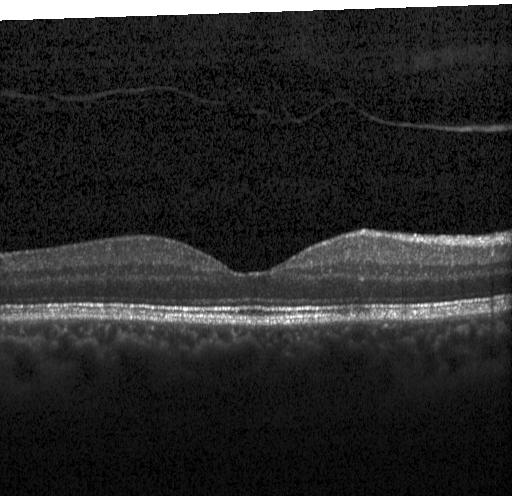

The scan shows no evidence of CNV, DME, or drusen.